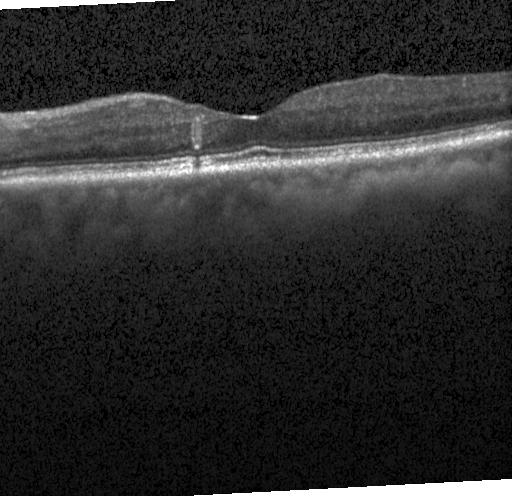
SD-OCT · fovea-centered · Heidelberg Spectralis · retinal OCT cross-section — Finding: no choroidal neovascularization, no diabetic macular edema, and no drusen.